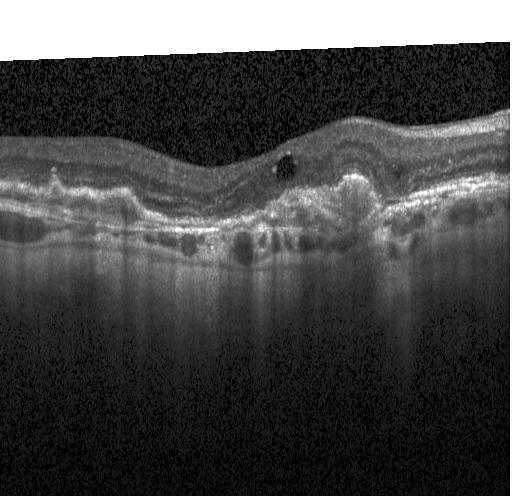
OCT scan showing CNV.